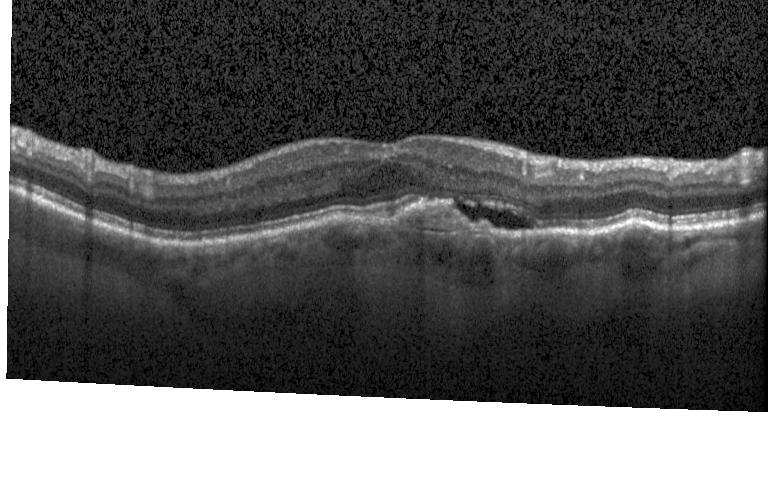
Retinal OCT B-scan; centered on the fovea; spectral-domain optical coherence tomography.
Finding: a choroidal neovascular membrane.